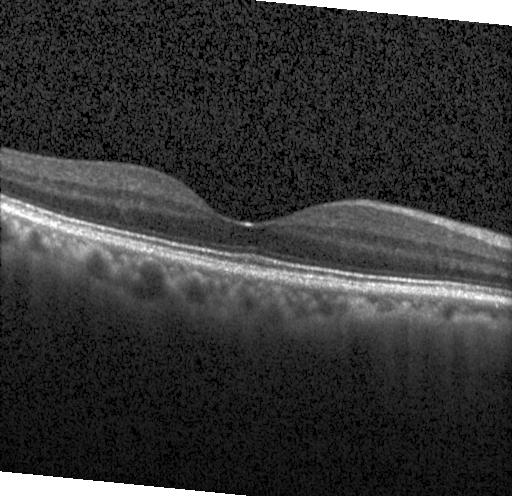
No evidence of CNV, DME, or drusen.